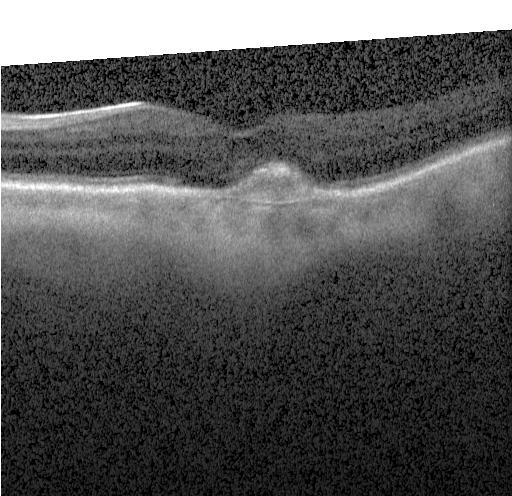 Optical coherence tomography scan; instrument: Heidelberg Spectralis; spectral-domain OCT. The scan shows a choroidal neovascular membrane.